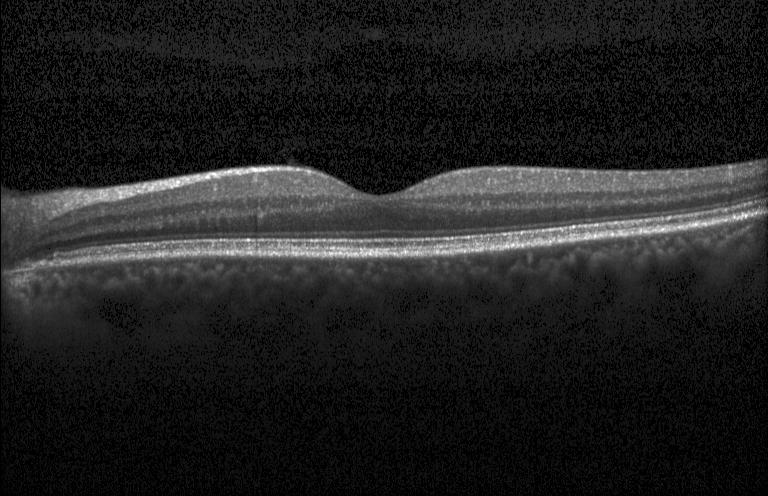

OCT line scan. The scan shows no choroidal neovascularization, no diabetic macular edema, and no drusen.